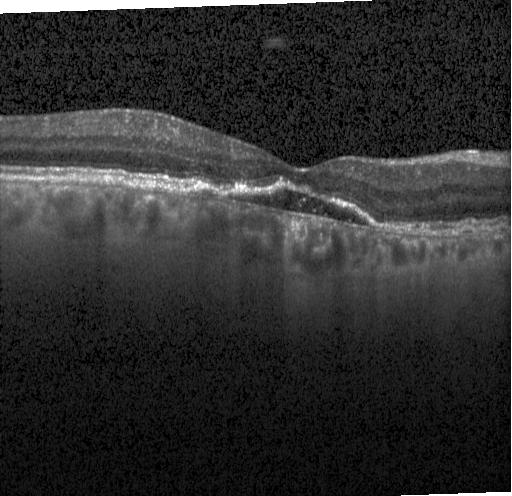
Macular scan · spectral-domain optical coherence tomography · acquired on a Heidelberg Spectralis · OCT line scan. This B-scan demonstrates a choroidal neovascular membrane.